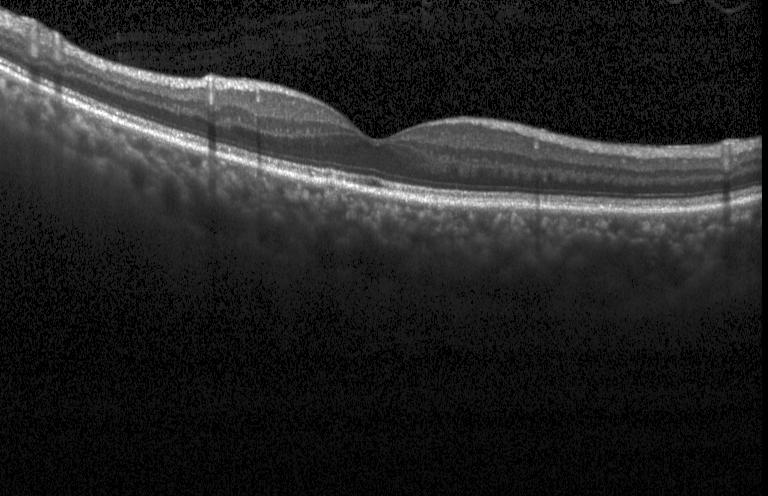

OCT line scan, through the macula
No evidence of choroidal neovascularization, diabetic macular edema, or drusen.